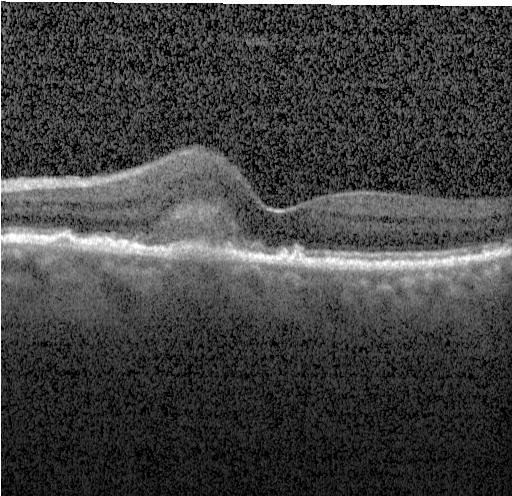 Instrument: Heidelberg Spectralis · retinal OCT B-scan · through the macula · spectral-domain optical coherence tomography. OCT finding: CNV.